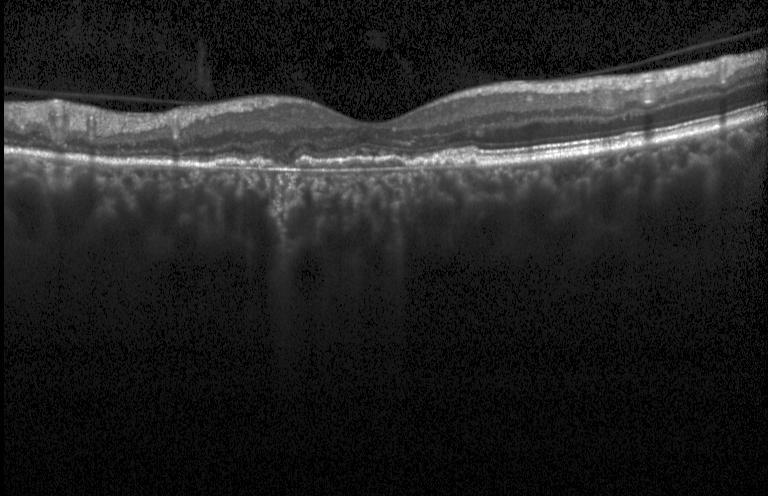 OCT finding: a choroidal neovascular membrane.